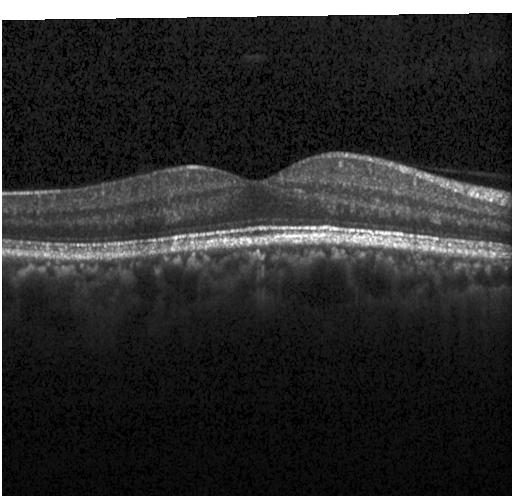 Spectral-domain OCT, optical coherence tomography scan, macular scan, Heidelberg Spectralis. Finding: no evidence of CNV, DME, or drusen.